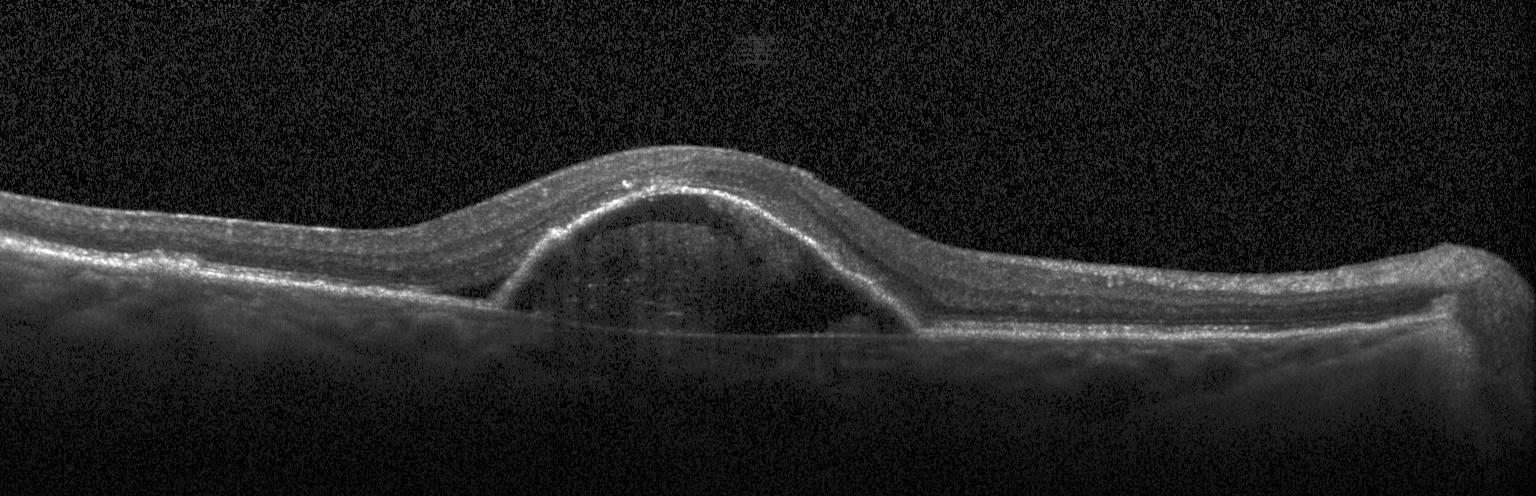

Spectral-domain OCT, horizontal scan through the fovea, Heidelberg Spectralis, optical coherence tomography scan — Dx: a choroidal neovascular membrane.